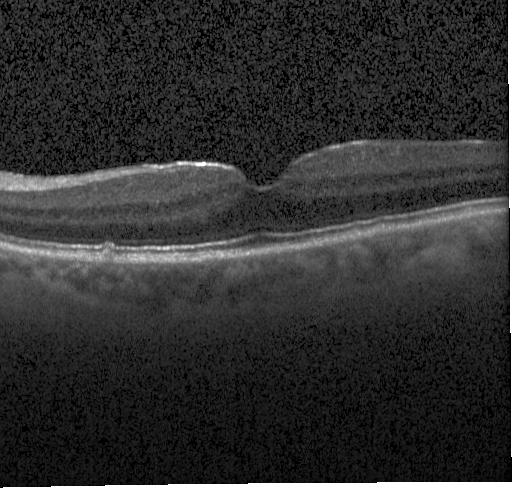 Retinal OCT B-scan — OCT finding: sub-RPE drusenoid deposits.